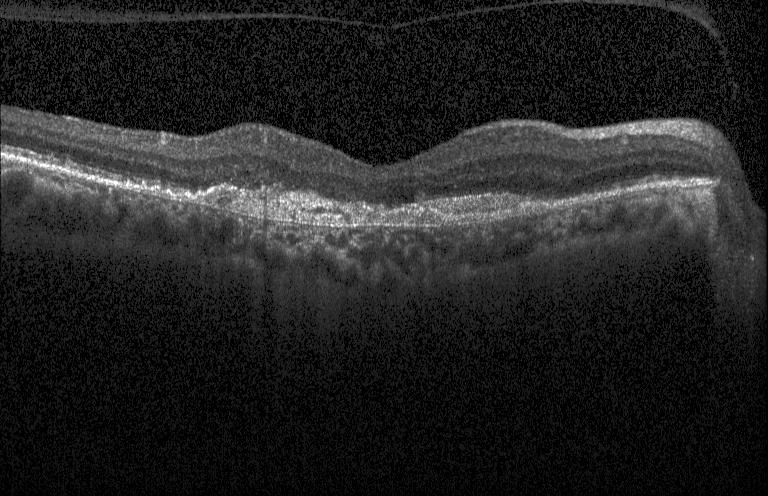 Retinal OCT B-scan. Fovea-centered. This B-scan demonstrates CNV.